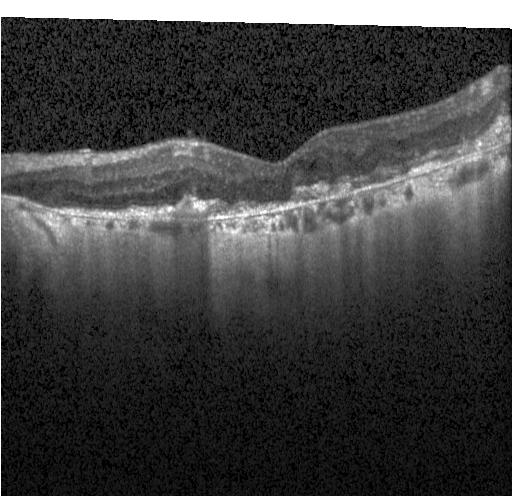

The scan shows choroidal neovascularization (CNV).